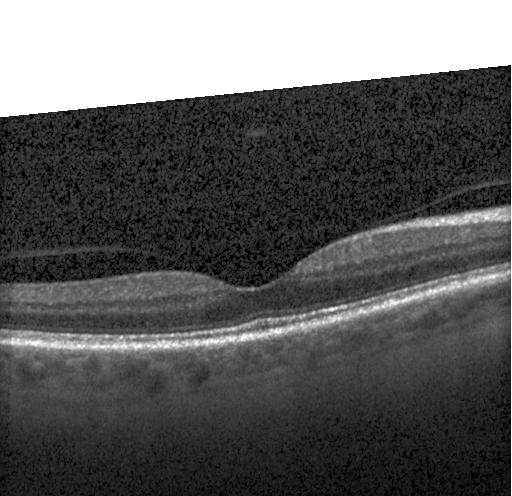
OCT line scan; through the macula.
Dx: no evidence of CNV, DME, or drusen.